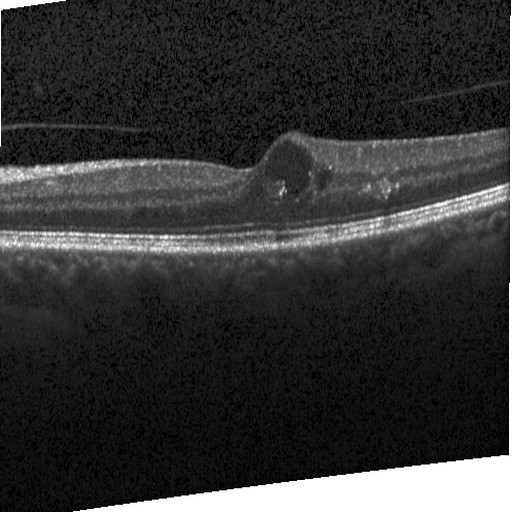
OCT B-scan · SD-OCT · macular scan
Dx: diabetic macular edema.